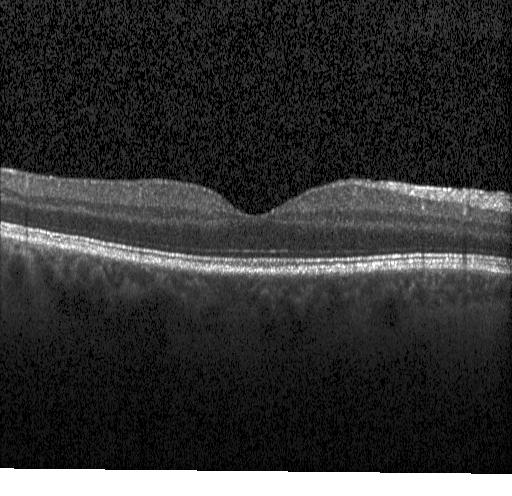

OCT scan showing no CNV, no DME, and no drusen.